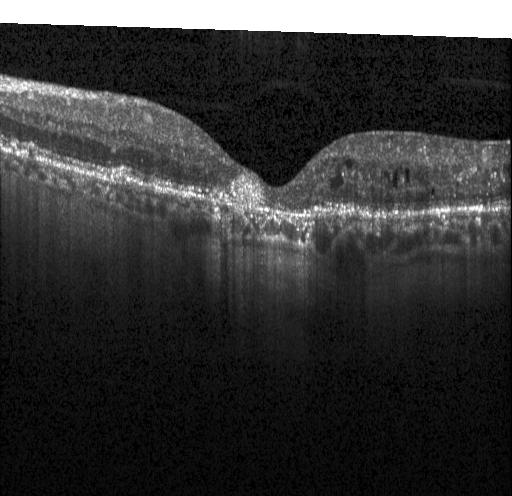
Diagnosis: choroidal neovascularization.